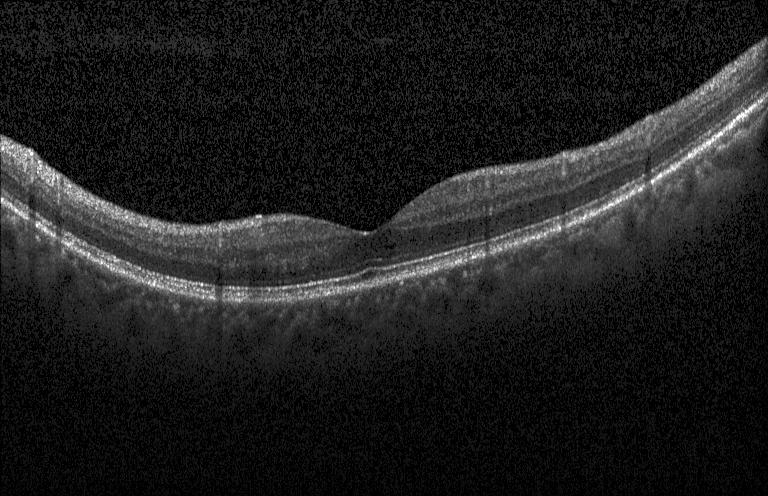
Optical coherence tomography scan — Finding: no choroidal neovascularization, diabetic macular edema, or drusen.